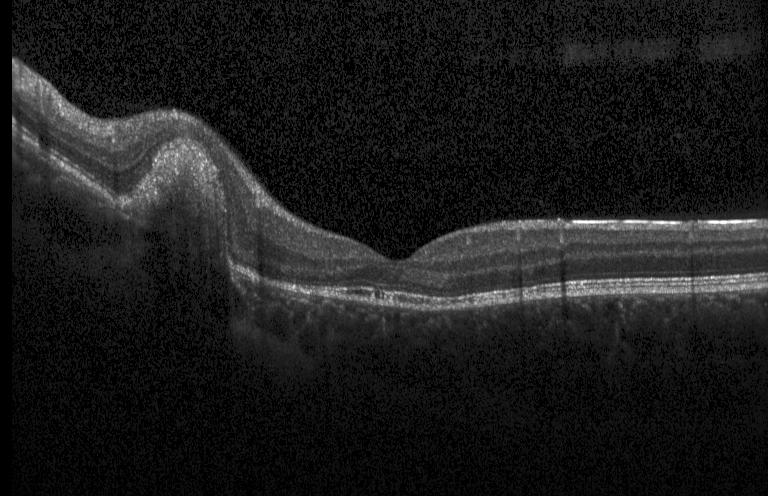

Retinal OCT cross-section
Impression: choroidal neovascularization (CNV).